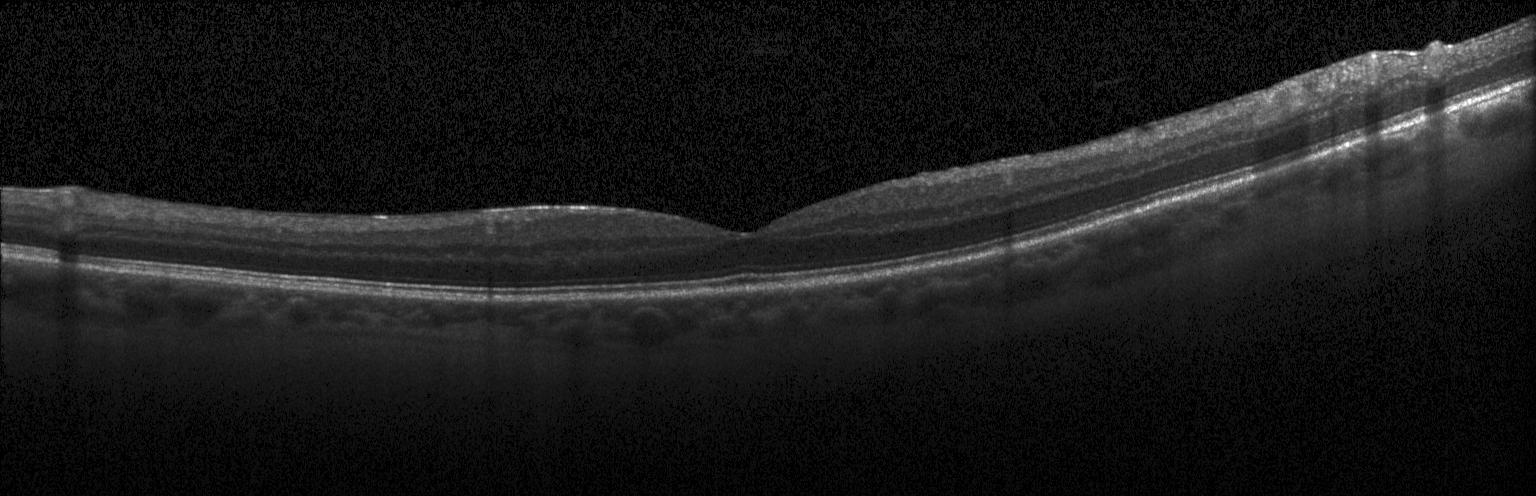
Macular scan; optical coherence tomography B-scan — No evidence of choroidal neovascularization, diabetic macular edema, or drusen.